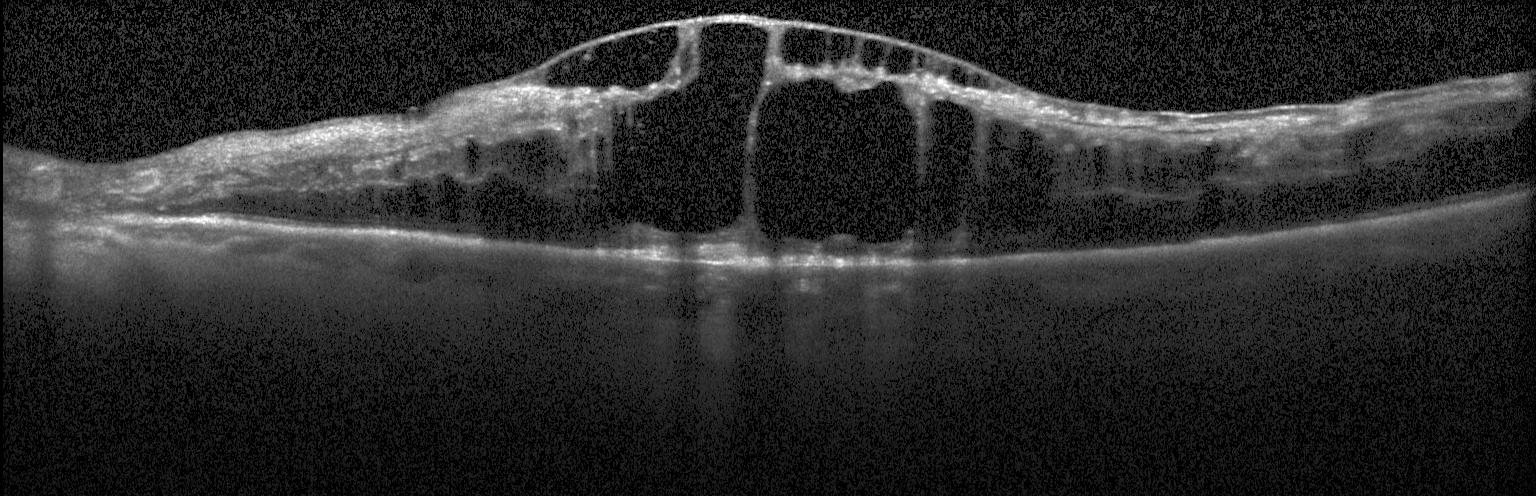

Dx: diabetic macular edema.